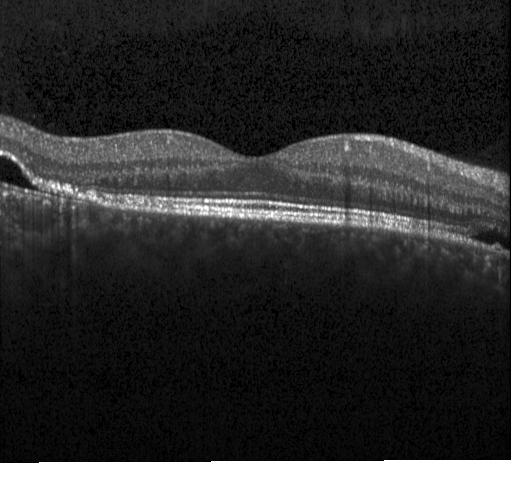

Retinal OCT cross-section.
Assessment: a choroidal neovascular membrane.